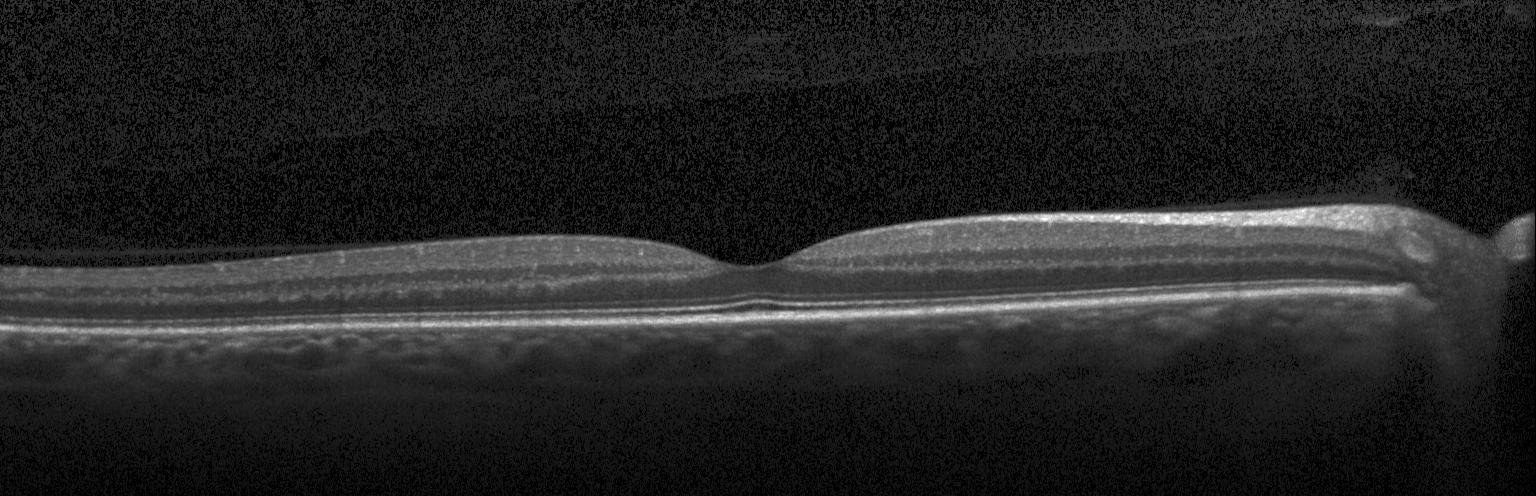
This B-scan demonstrates neither CNV, DME, nor drusen.